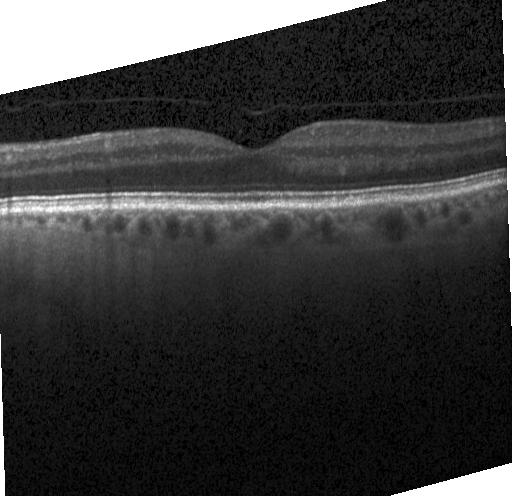
Retinal OCT cross-section, acquired on a Heidelberg Spectralis, spectral-domain OCT.
Assessment: no choroidal neovascularization, diabetic macular edema, or drusen.